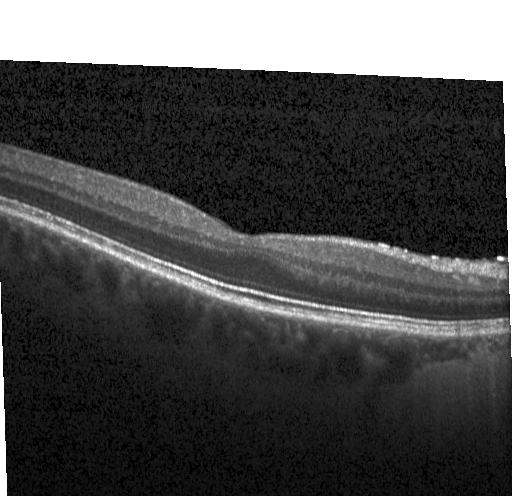

Finding: no evidence of CNV, DME, or drusen.